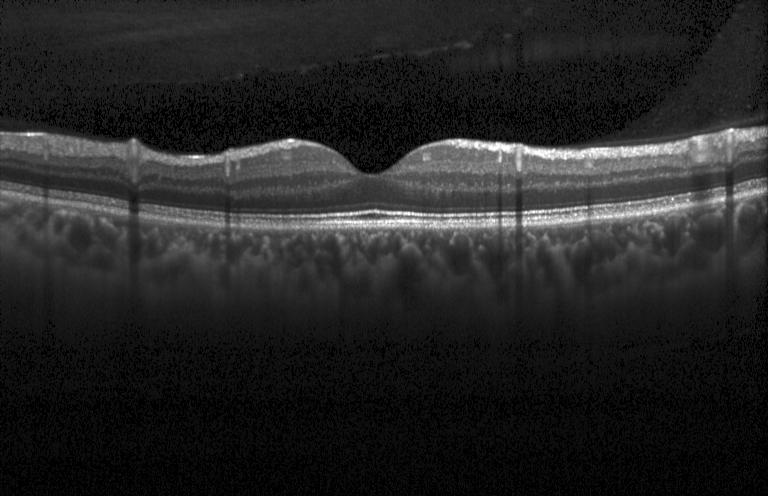

Finding: no choroidal neovascularization, diabetic macular edema, or drusen.